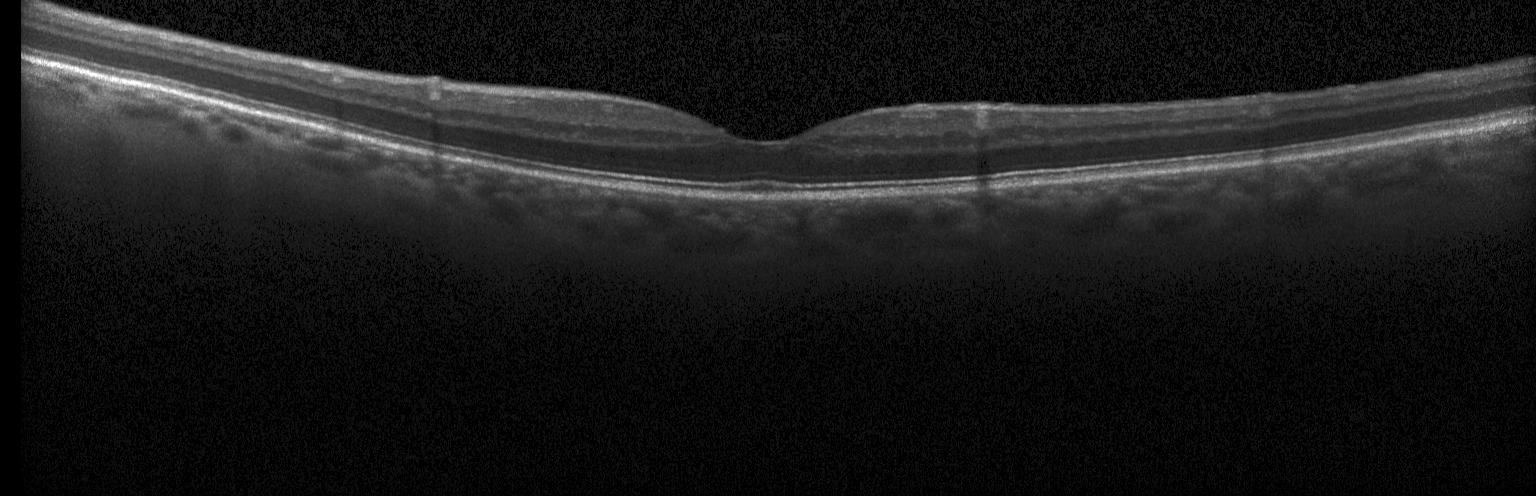

Macular OCT demonstrating no choroidal neovascularization, diabetic macular edema, or drusen.